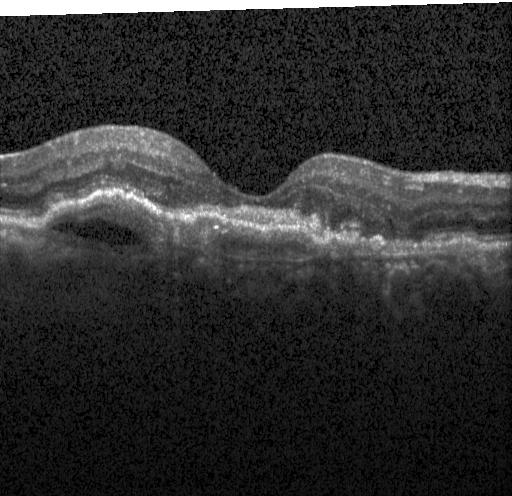
OCT B-scan showing a choroidal neovascular membrane.